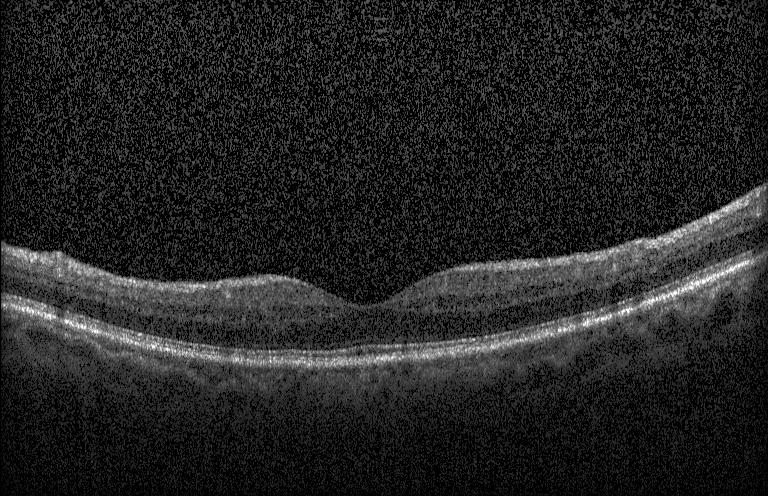 Assessment: no evidence of choroidal neovascularization, diabetic macular edema, or drusen.